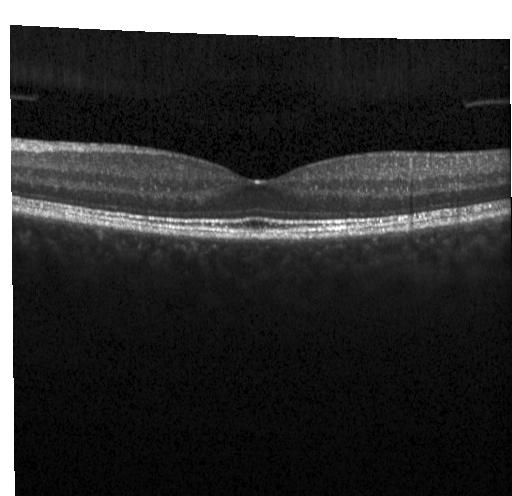 Acquired on a Heidelberg Spectralis; through the macula; retinal OCT cross-section.
The scan shows no choroidal neovascularization, no diabetic macular edema, and no drusen.